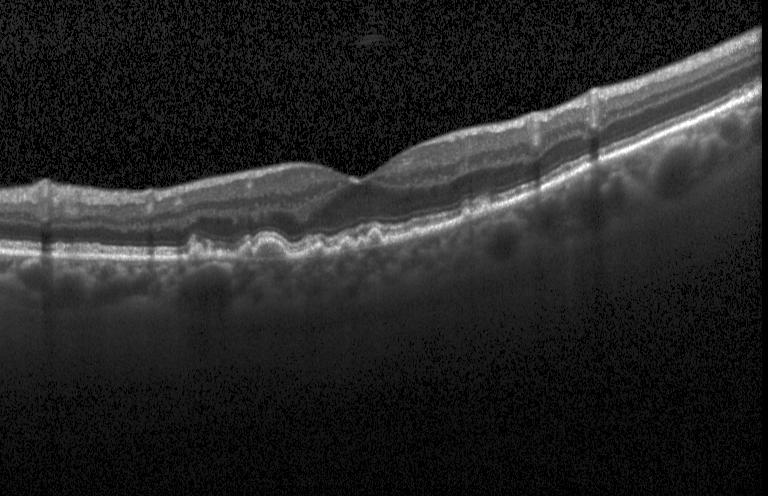 The scan shows multiple drusen.